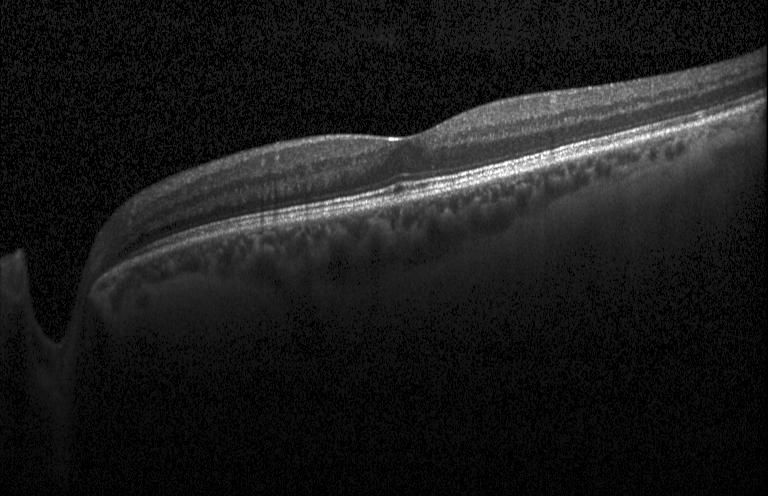

Spectral-domain optical coherence tomography, retinal OCT cross-section, horizontal scan through the fovea
This B-scan demonstrates no evidence of choroidal neovascularization, diabetic macular edema, or drusen.